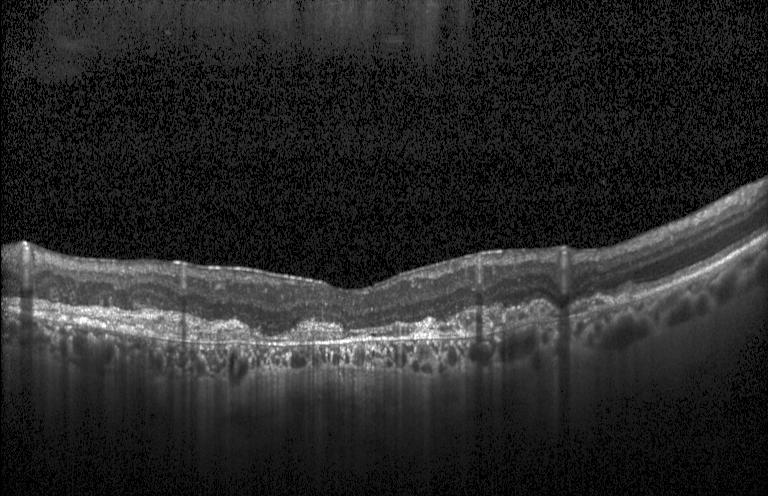 Heidelberg Spectralis. SD-OCT. Macular scan. Retinal OCT cross-section. This B-scan demonstrates CNV.